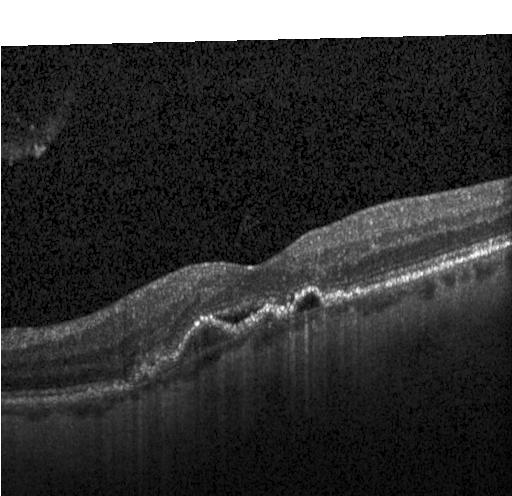

Macular OCT: choroidal neovascularization (CNV).